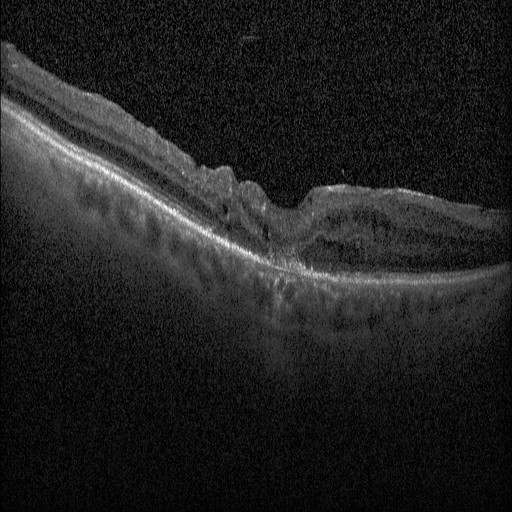

Finding: DME.